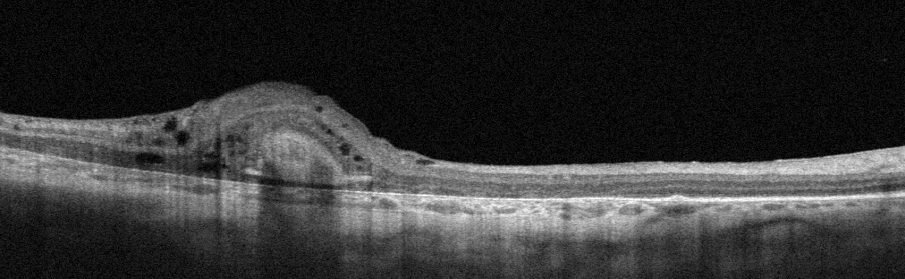
OCT line scan.
Finding: age-related macular degeneration.